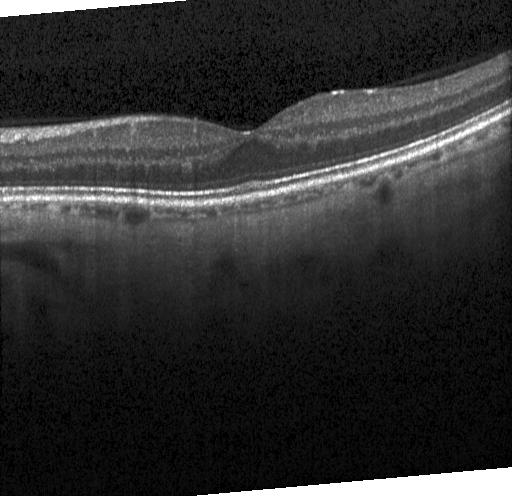

Retinal OCT B-scan — OCT finding: neither choroidal neovascularization, diabetic macular edema, nor drusen.